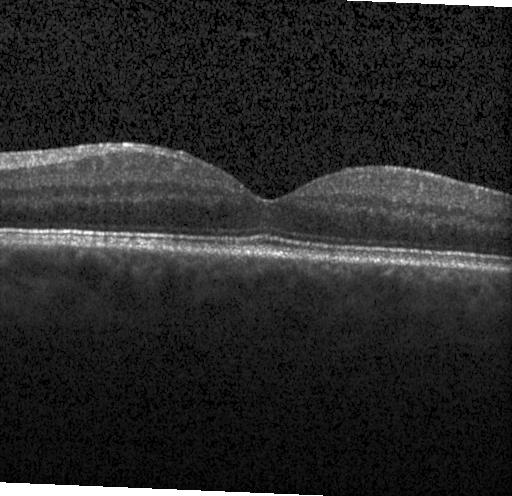
Macular scan; optical coherence tomography B-scan; SD-OCT.
Finding: no choroidal neovascularization, no diabetic macular edema, and no drusen.